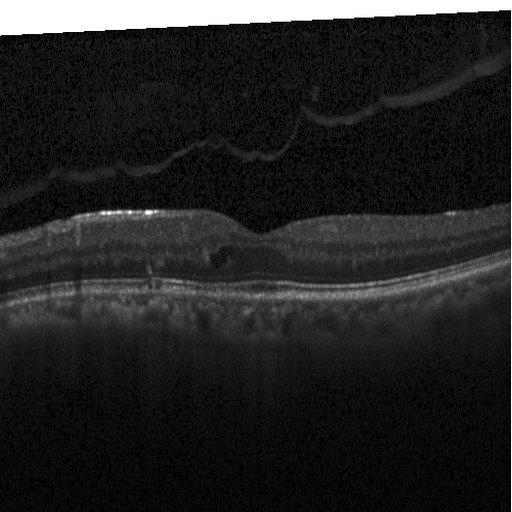 OCT B-scan — Diabetic macular edema (DME).